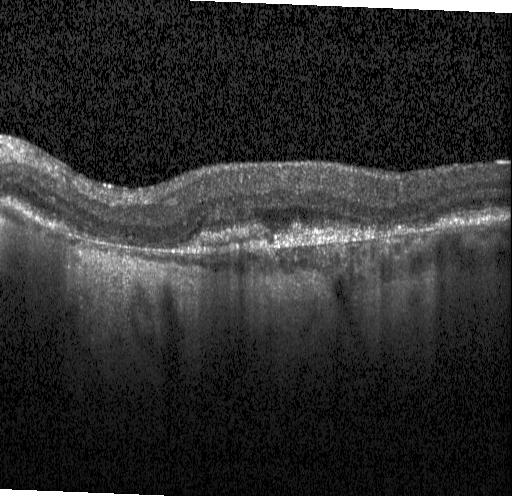

Heidelberg Spectralis · spectral-domain OCT · optical coherence tomography scan — Dx: a choroidal neovascular membrane.